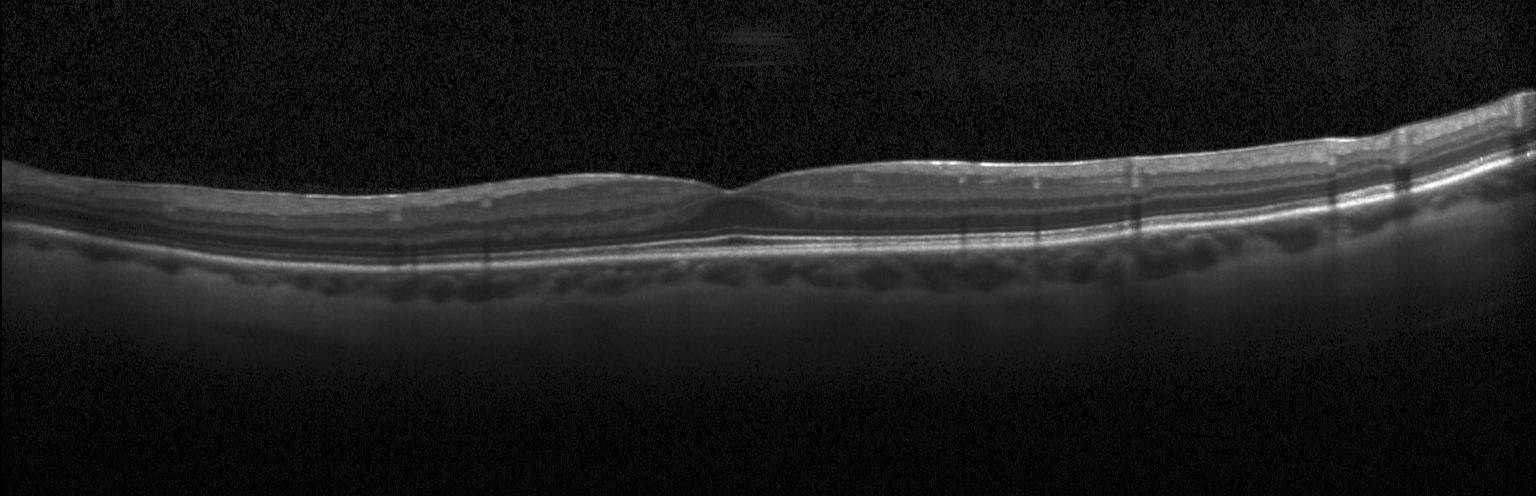

Heidelberg Spectralis, OCT line scan.
Diagnosis: neither choroidal neovascularization, diabetic macular edema, nor drusen.